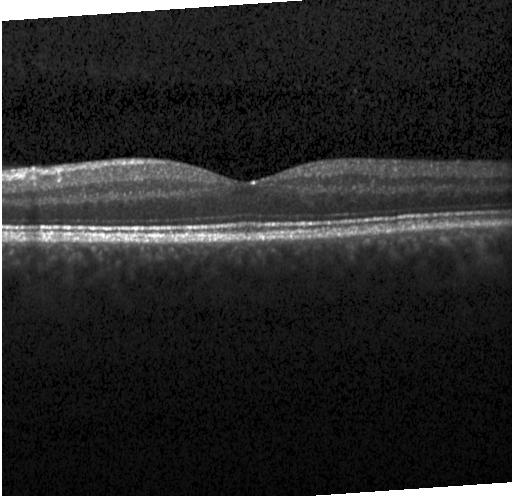 Optical coherence tomography scan
Dx: no CNV, no DME, and no drusen.